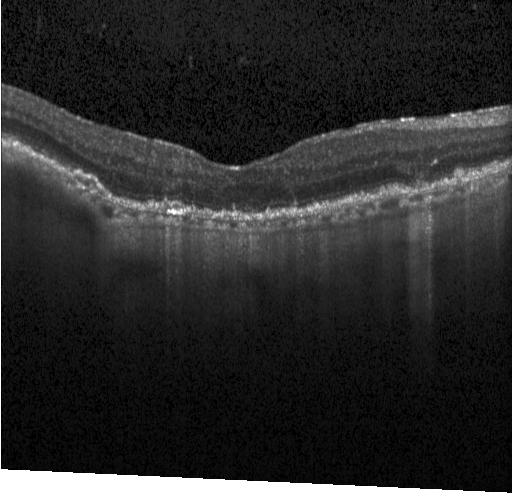

OCT finding: a choroidal neovascular membrane.